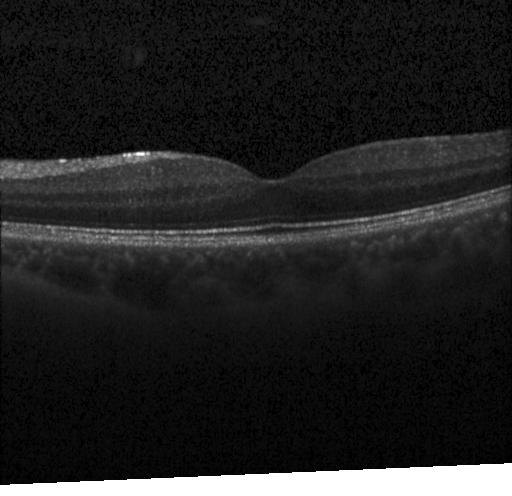

Impression: no evidence of choroidal neovascularization, diabetic macular edema, or drusen.